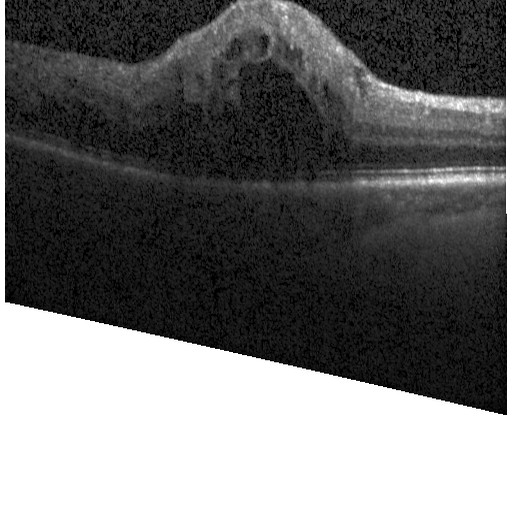

Macular scan; spectral-domain optical coherence tomography; retinal OCT B-scan. Impression: diabetic macular edema (DME).